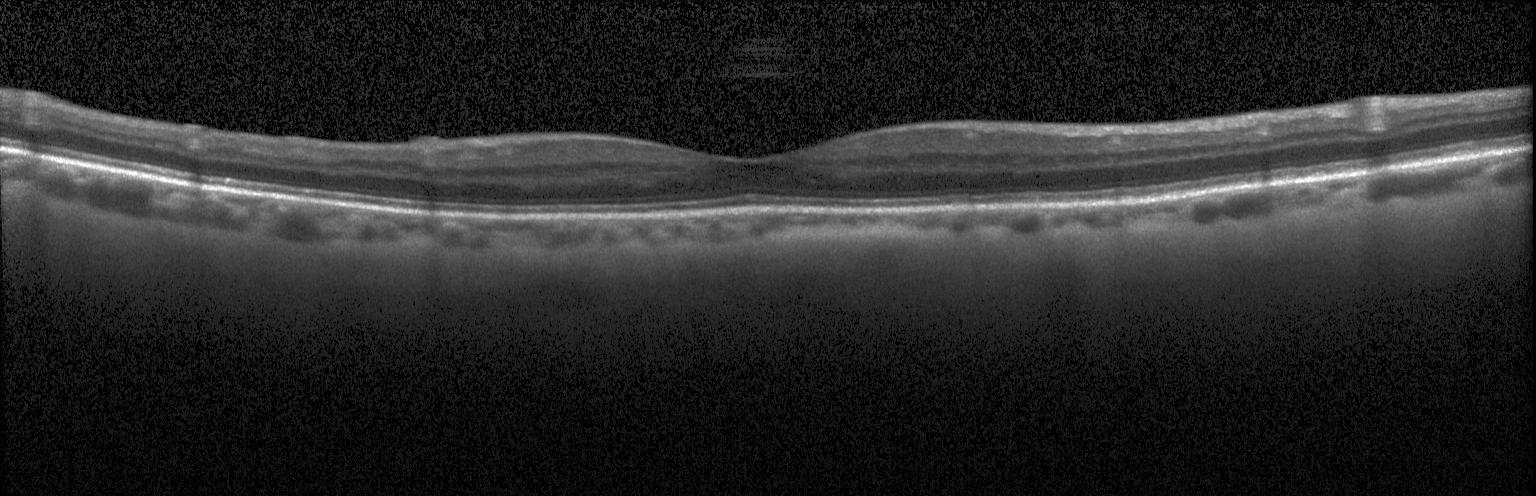

Impression: no choroidal neovascularization, diabetic macular edema, or drusen.